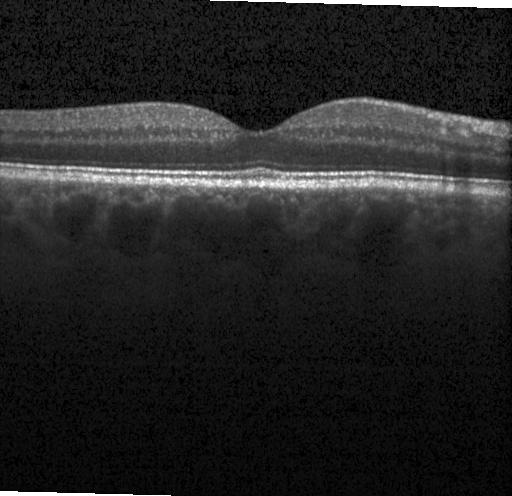 Macular OCT: no choroidal neovascularization, no diabetic macular edema, and no drusen.